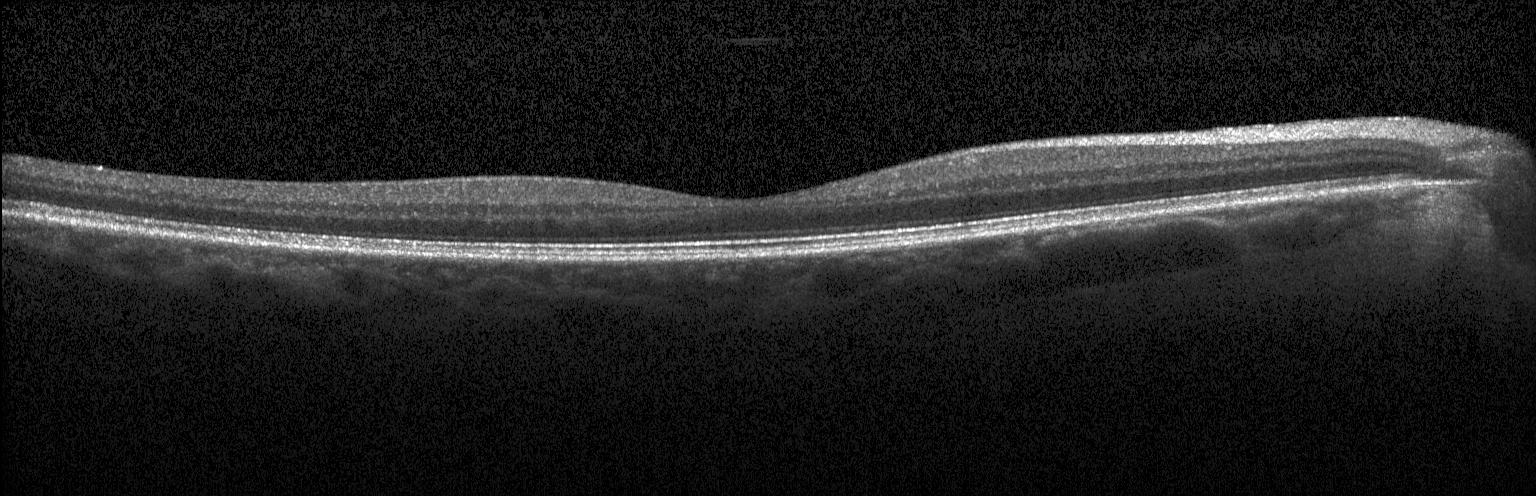

Spectral-domain OCT, centered on the fovea, acquired on a Heidelberg Spectralis, OCT B-scan — The scan shows neither choroidal neovascularization, diabetic macular edema, nor drusen.